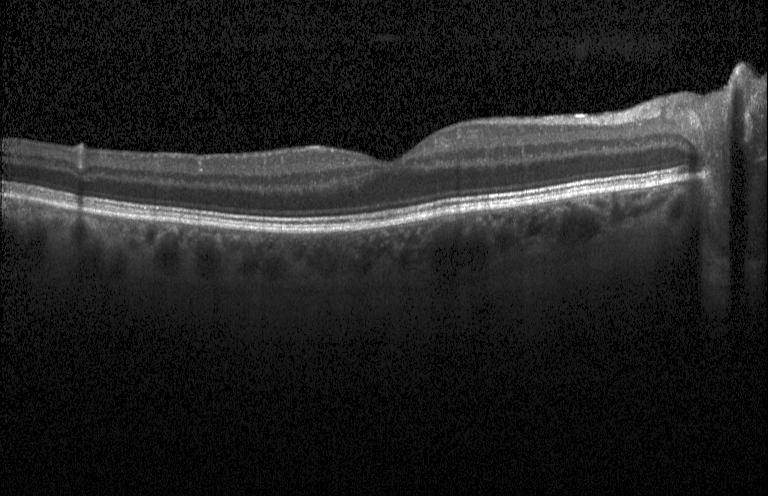 OCT B-scan · SD-OCT · macular scan · acquired on a Heidelberg Spectralis.
Diagnosis: no choroidal neovascularization, no diabetic macular edema, and no drusen.